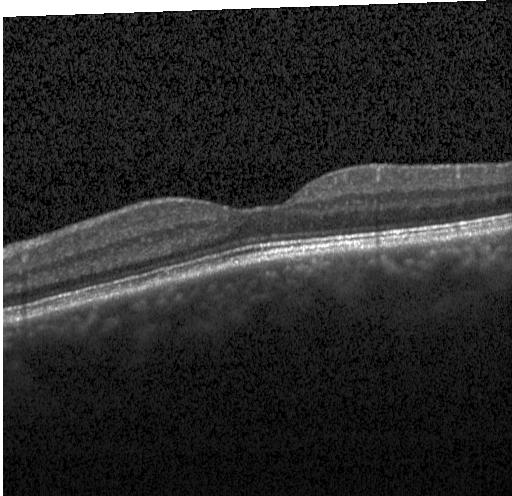
OCT line scan — Diagnosis: no evidence of CNV, DME, or drusen.